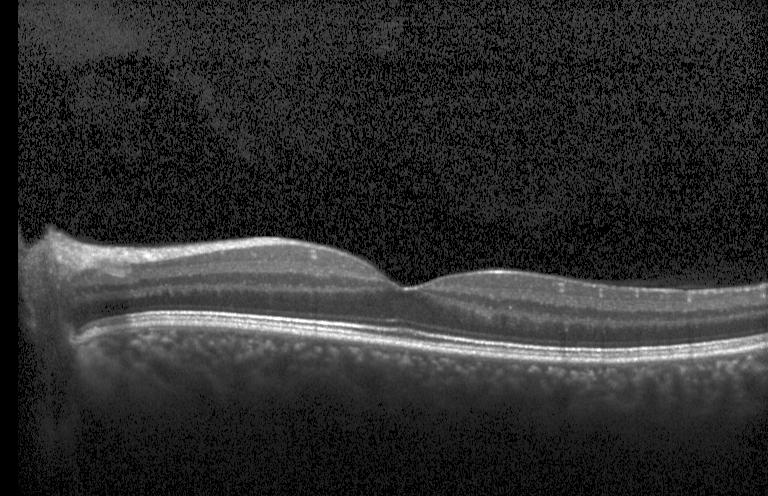
Macular OCT demonstrating neither CNV, DME, nor drusen.